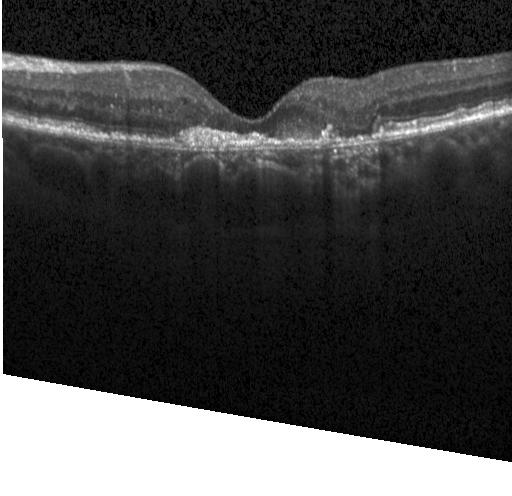

Horizontal scan through the fovea. OCT B-scan. Impression: choroidal neovascularization (CNV).